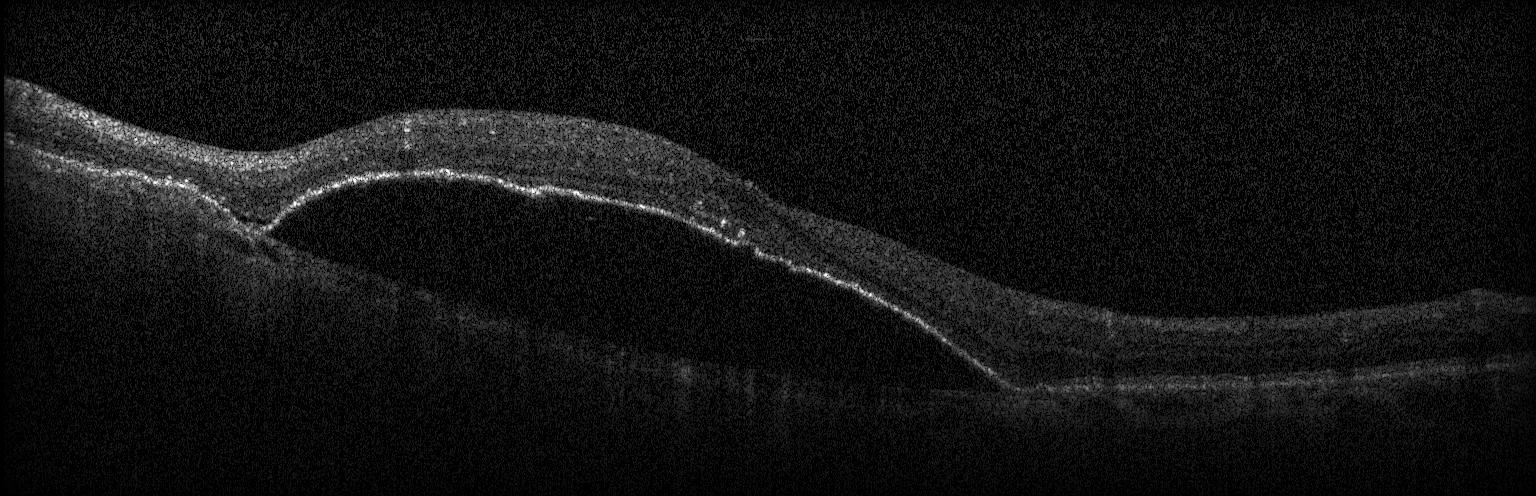

Choroidal neovascularization.